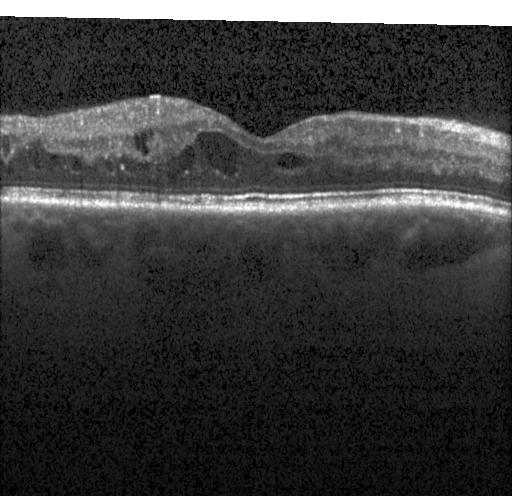 Macular OCT: diabetic macular edema (DME).